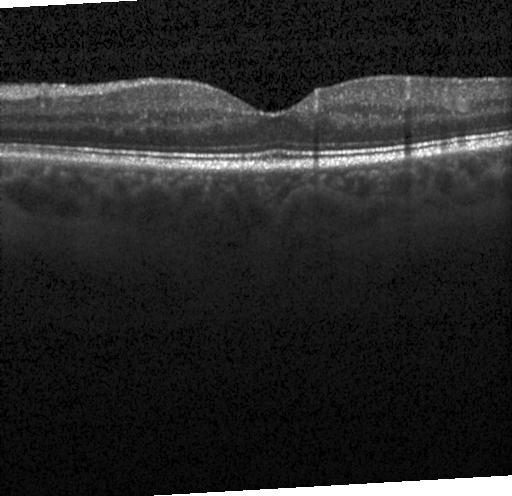 Instrument: Heidelberg Spectralis. OCT line scan. Horizontal scan through the fovea.
Finding: no CNV, no DME, and no drusen.